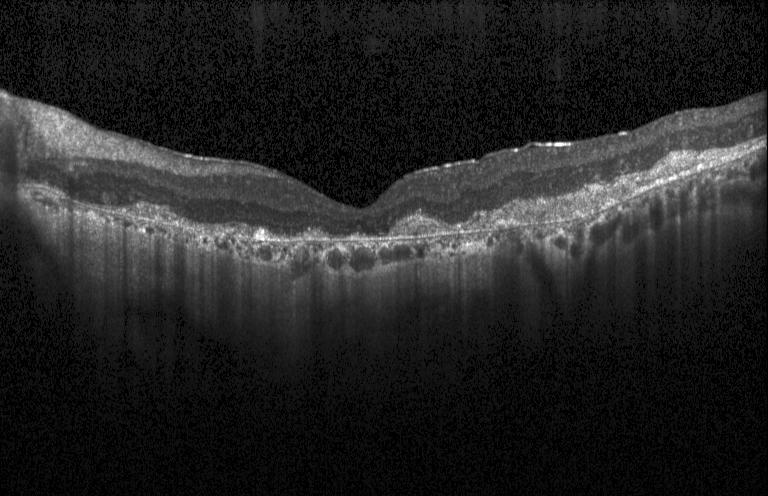

OCT finding: a choroidal neovascular membrane.